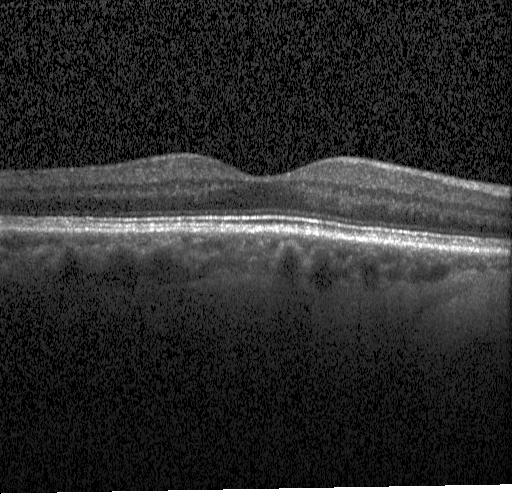

SD-OCT. Retinal OCT cross-section — The scan shows no CNV, DME, or drusen.